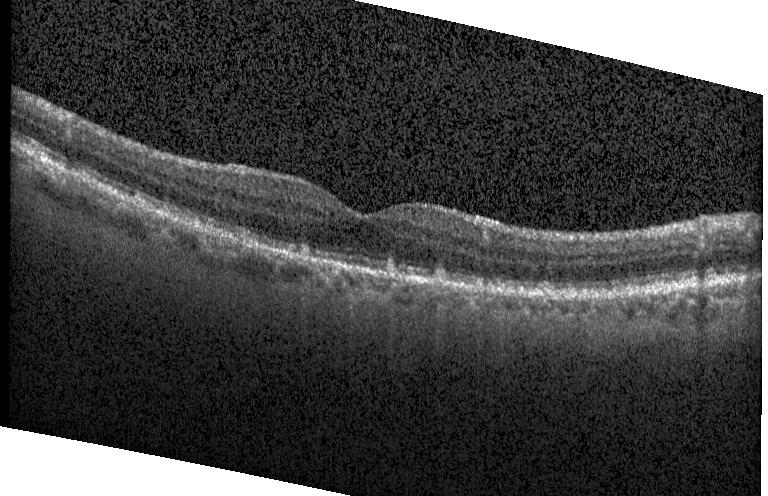 Spectral-domain OCT, instrument: Heidelberg Spectralis, optical coherence tomography scan, horizontal scan through the fovea — Impression: drusen.